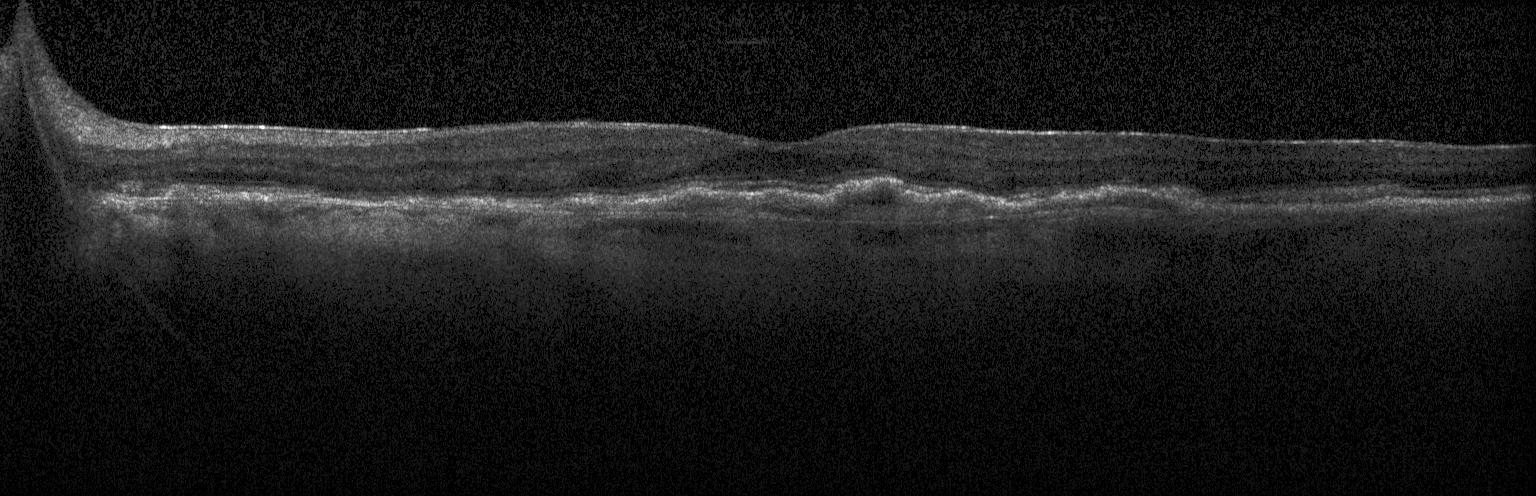

OCT line scan. SD-OCT. Fovea-centered. Heidelberg Spectralis OCT system.
Macular OCT: choroidal neovascularization.